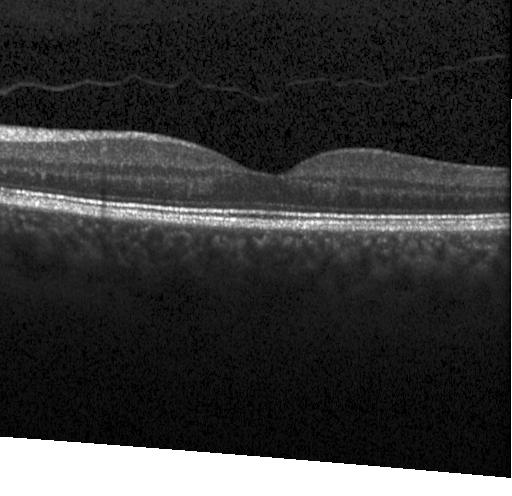
Diagnosis: neither choroidal neovascularization, diabetic macular edema, nor drusen.